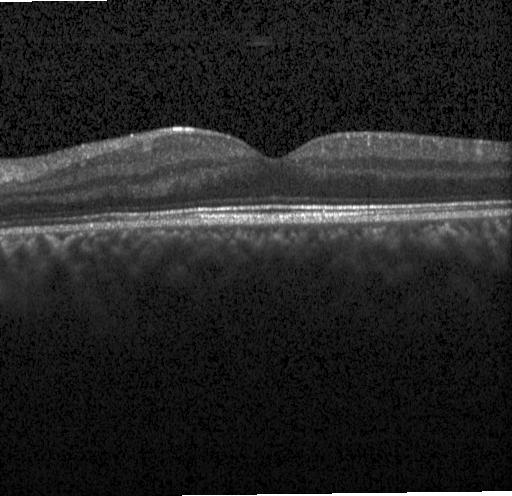

SD-OCT, retinal OCT cross-section.
Diagnosis: no choroidal neovascularization, no diabetic macular edema, and no drusen.